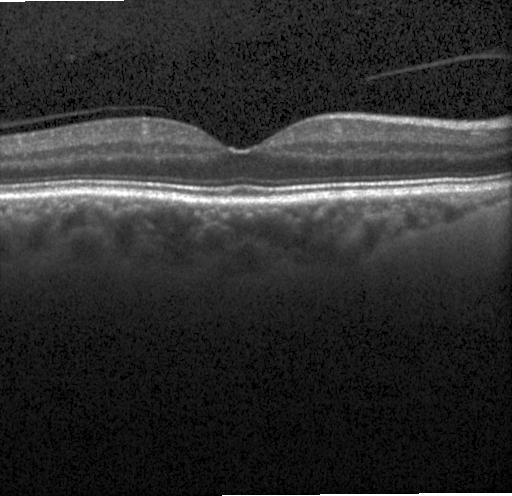

Retinal OCT cross-section showing no evidence of choroidal neovascularization, diabetic macular edema, or drusen.